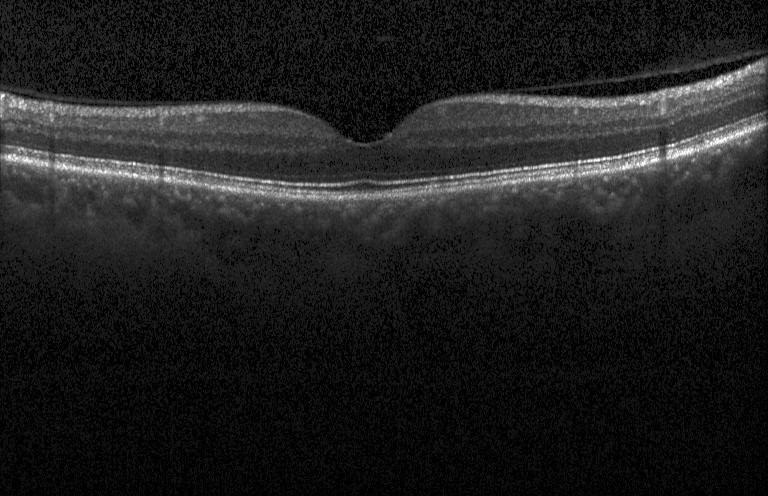 Impression: neither choroidal neovascularization, diabetic macular edema, nor drusen.